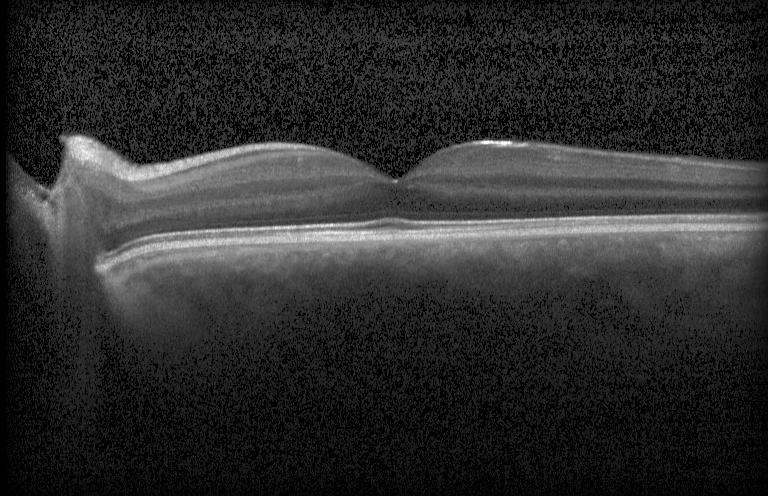 Optical coherence tomography B-scan. Impression: no choroidal neovascularization, diabetic macular edema, or drusen.